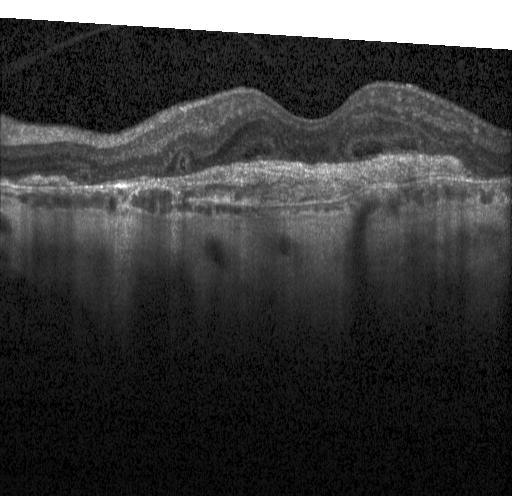

Spectral-domain optical coherence tomography; Heidelberg Spectralis; through the macula; optical coherence tomography B-scan
Finding: choroidal neovascularization (CNV).